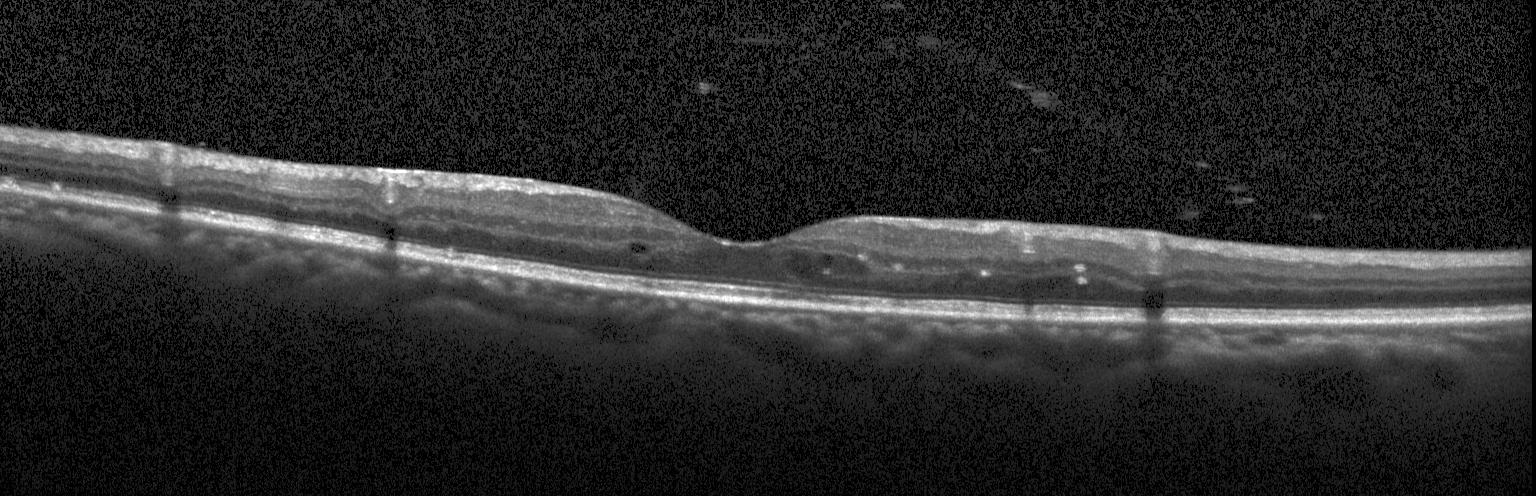

Finding: diabetic macular edema (DME).